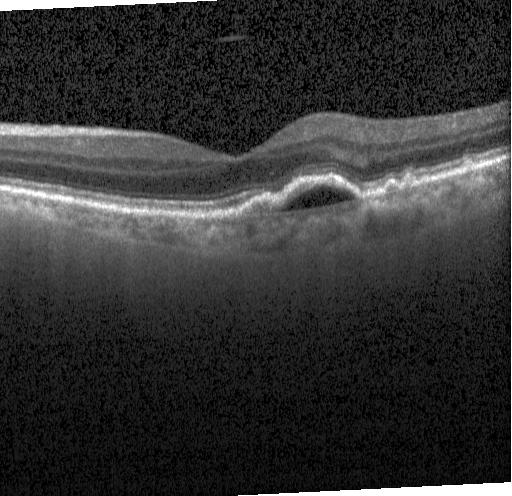 Macular scan, retinal OCT B-scan, spectral-domain optical coherence tomography
Dx: choroidal neovascularization (CNV).